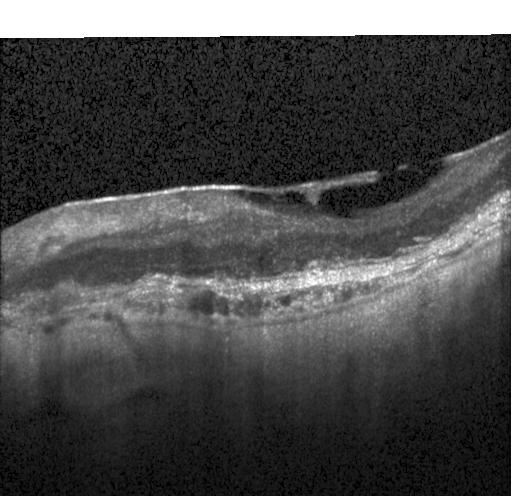
Finding: a choroidal neovascular membrane.